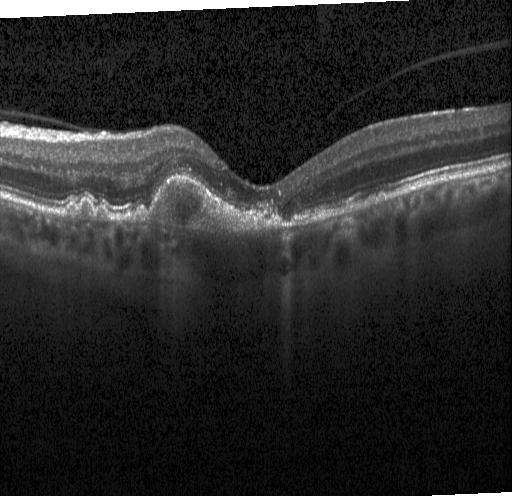
Retinal OCT B-scan · Heidelberg Spectralis OCT system — Impression: a choroidal neovascular membrane.